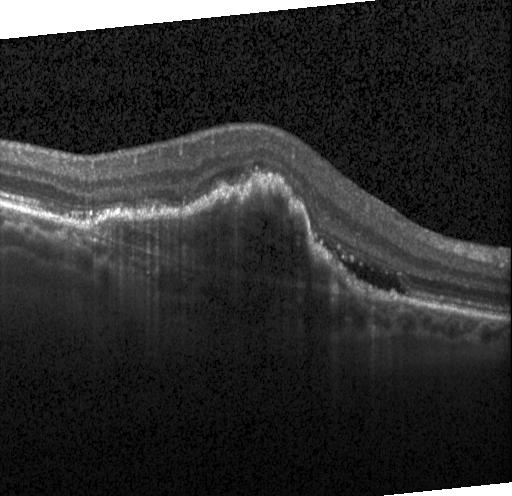 Spectral-domain OCT. OCT line scan. Centered on the fovea. Heidelberg Spectralis
Finding: choroidal neovascularization (CNV).